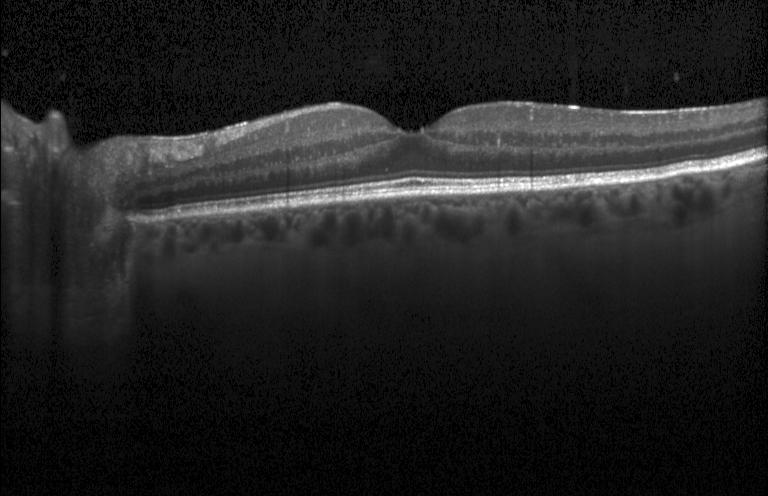 Acquired on a Heidelberg Spectralis; optical coherence tomography B-scan; horizontal scan through the fovea
Finding: no evidence of CNV, DME, or drusen.